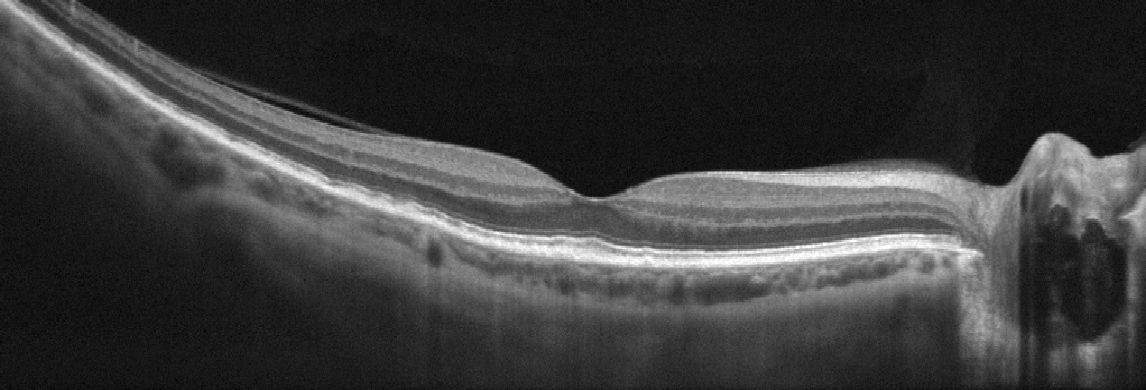
Optical coherence tomography scan; fovea-centered
Dx: AMD.